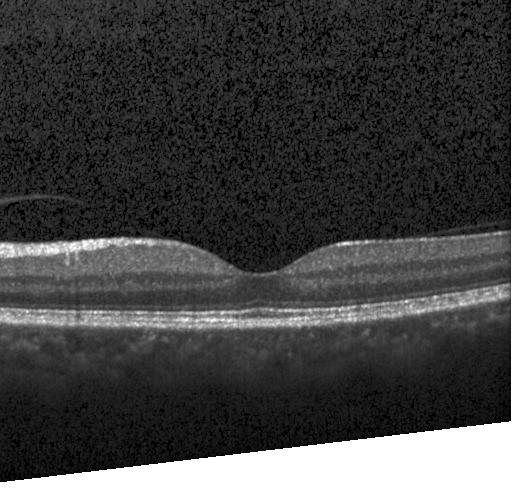 Impression: neither choroidal neovascularization, diabetic macular edema, nor drusen.